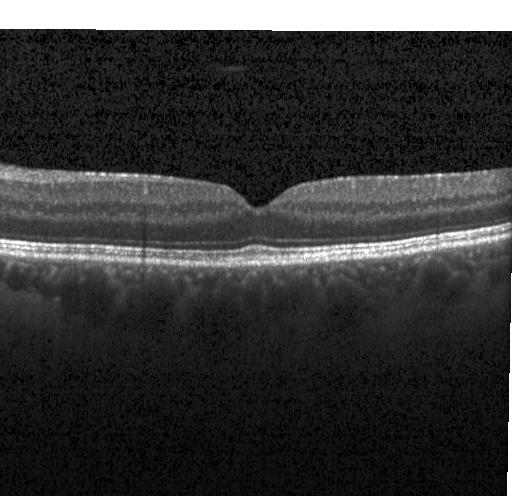 Macular OCT demonstrating neither choroidal neovascularization, diabetic macular edema, nor drusen.